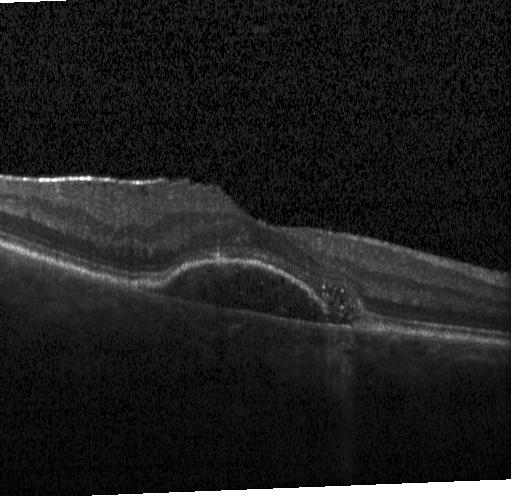 Spectral-domain optical coherence tomography · OCT B-scan · instrument: Heidelberg Spectralis. This B-scan demonstrates a choroidal neovascular membrane.